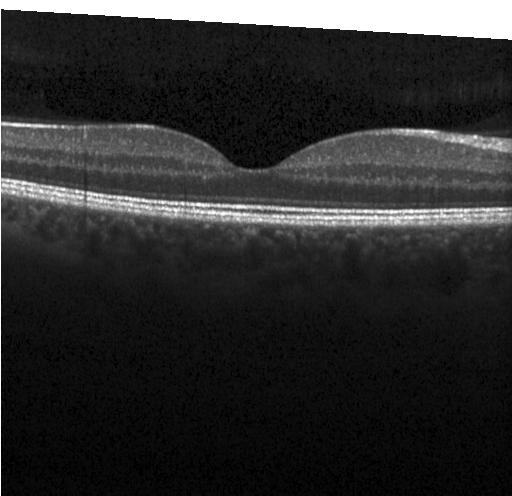 Spectral-domain OCT · horizontal scan through the fovea · optical coherence tomography B-scan · instrument: Heidelberg Spectralis.
OCT finding: no CNV, DME, or drusen.